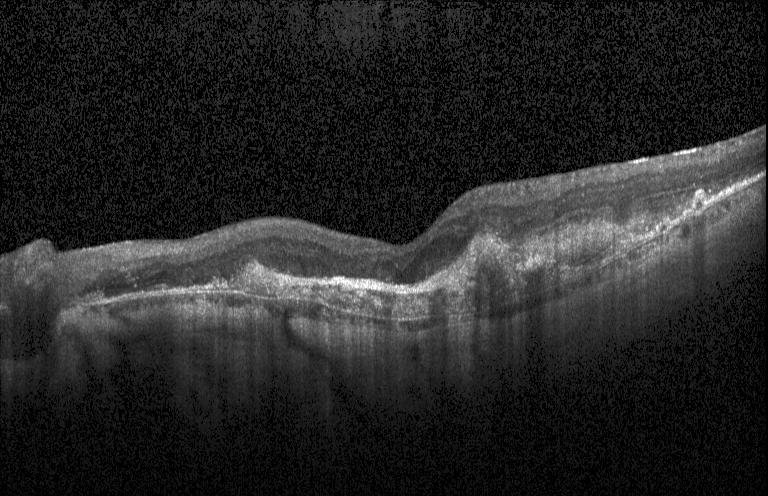 OCT scan showing choroidal neovascularization.